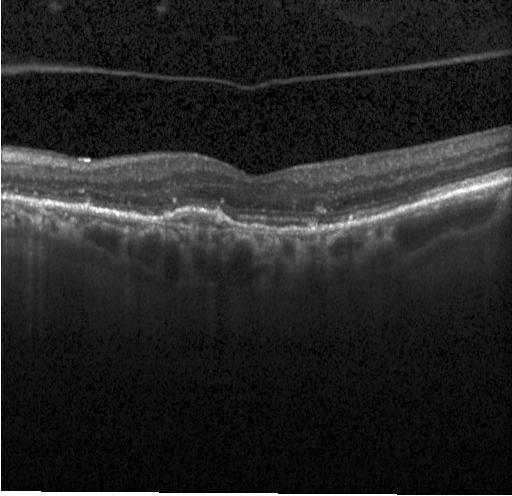 Retinal OCT cross-section. Fovea-centered. Heidelberg Spectralis. SD-OCT — Dx: choroidal neovascularization (CNV).